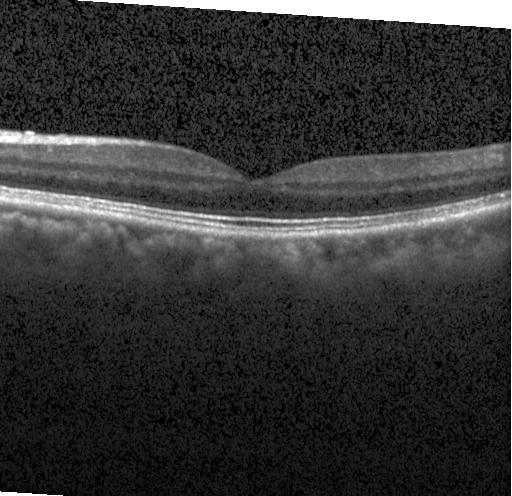 OCT scan showing neither choroidal neovascularization, diabetic macular edema, nor drusen.